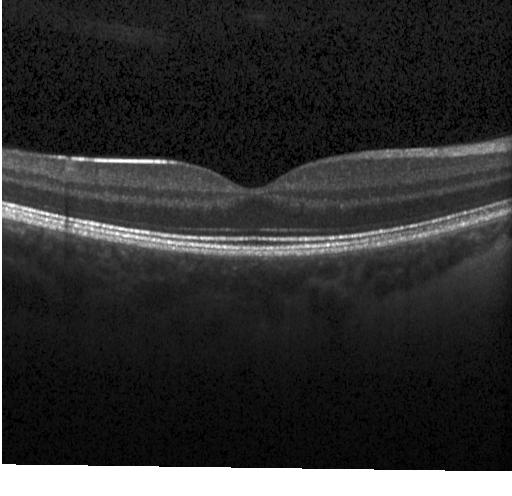 Optical coherence tomography scan. Diagnosis: no choroidal neovascularization, diabetic macular edema, or drusen.